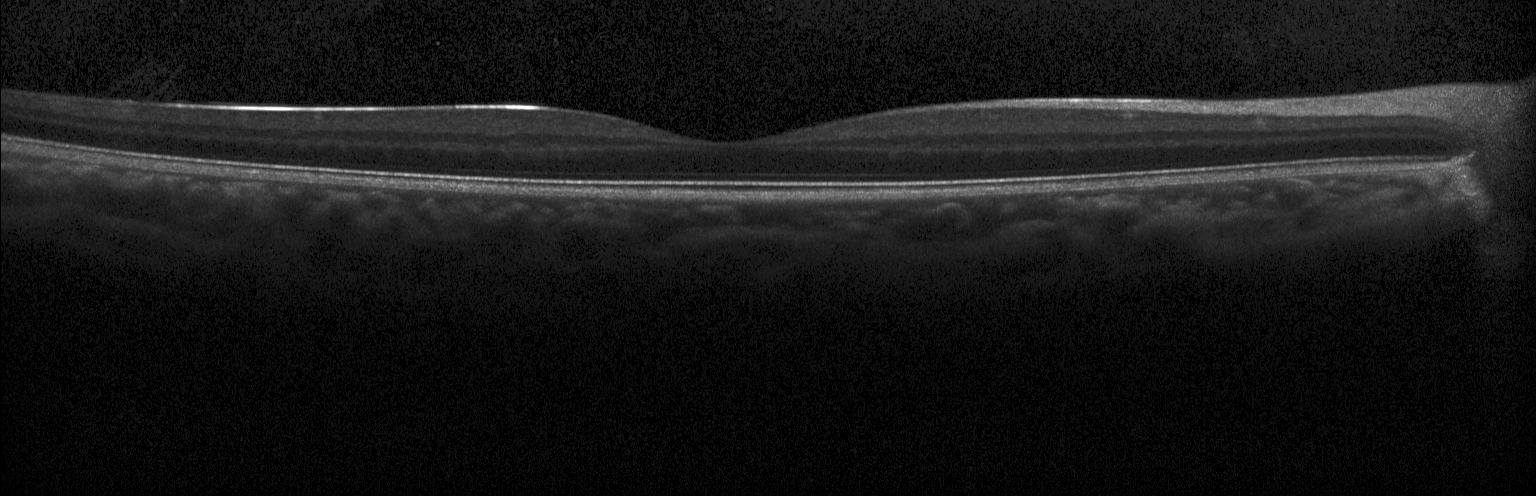

Finding: no evidence of choroidal neovascularization, diabetic macular edema, or drusen.